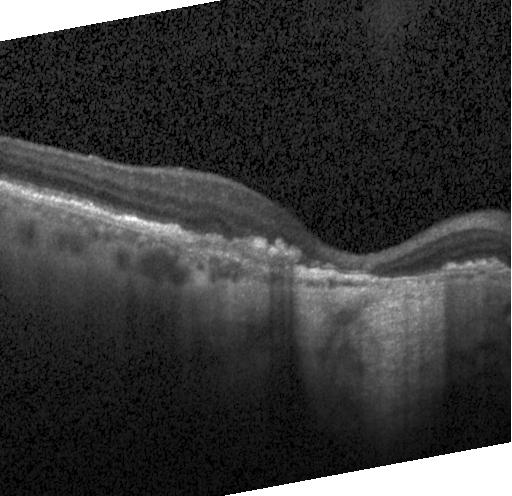 Retinal OCT B-scan, spectral-domain OCT. Impression: a choroidal neovascular membrane.